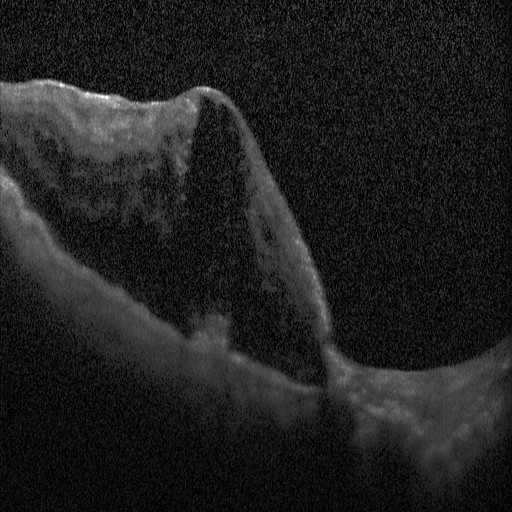 Finding: diabetic macular edema.